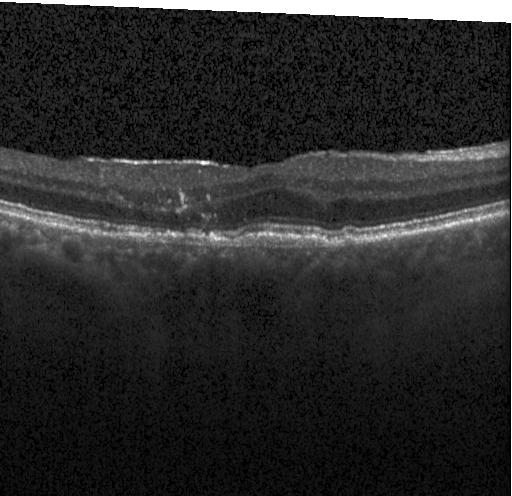
Dx: CNV.